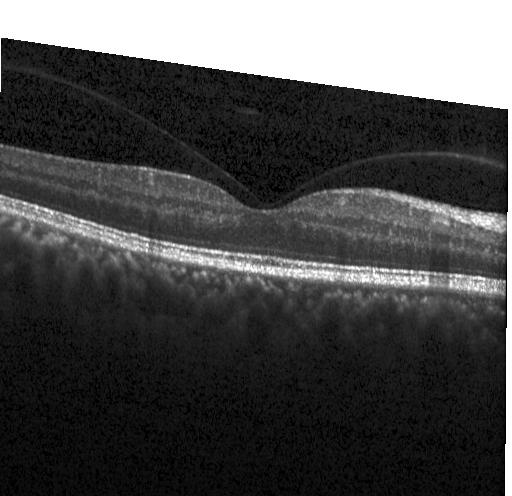
Optical coherence tomography B-scan.
Impression: no CNV, no DME, and no drusen.